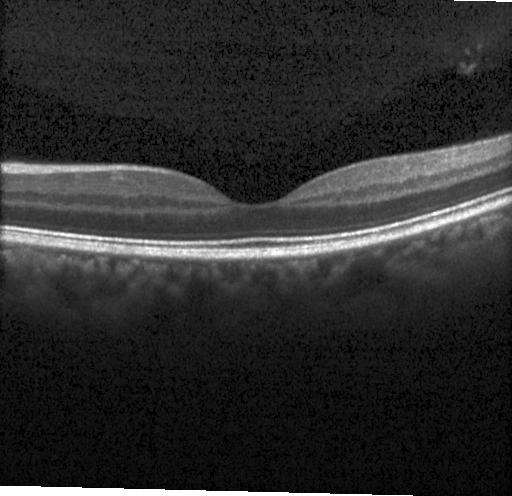

No CNV, DME, or drusen.